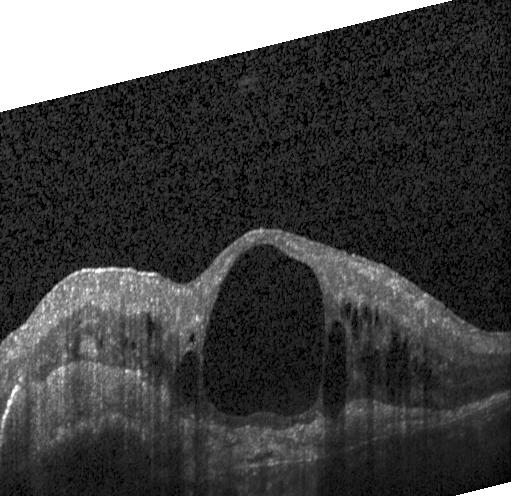 Optical coherence tomography scan
Finding: choroidal neovascularization.